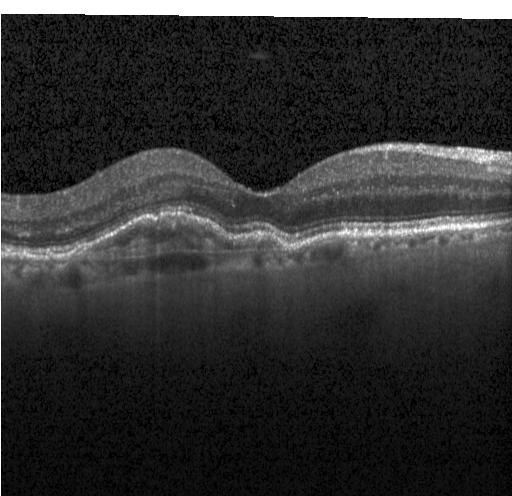

Optical coherence tomography scan. Heidelberg Spectralis. Assessment: a choroidal neovascular membrane.